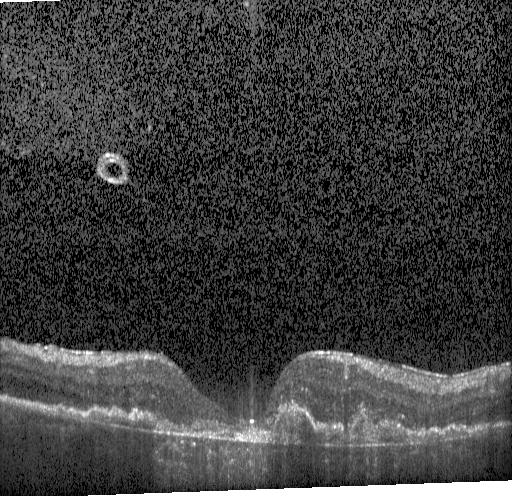
Spectral-domain OCT. Fovea-centered. Optical coherence tomography scan. Instrument: Heidelberg Spectralis — Assessment: CNV.